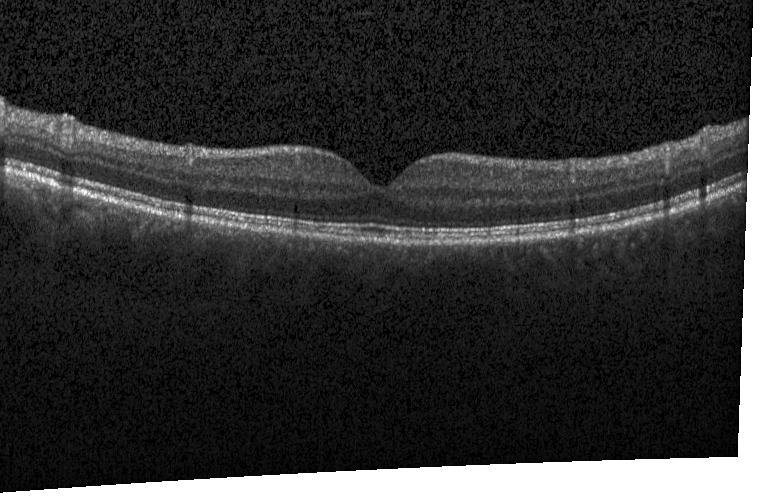
Optical coherence tomography B-scan. OCT finding: neither choroidal neovascularization, diabetic macular edema, nor drusen.